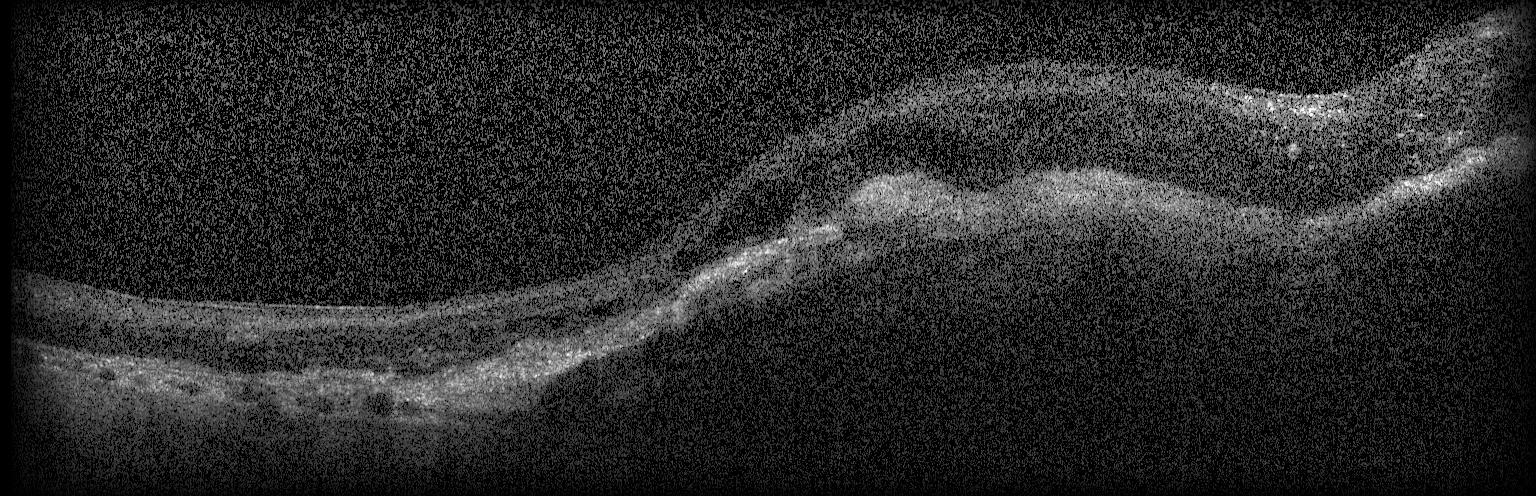 Diagnosis: CNV.